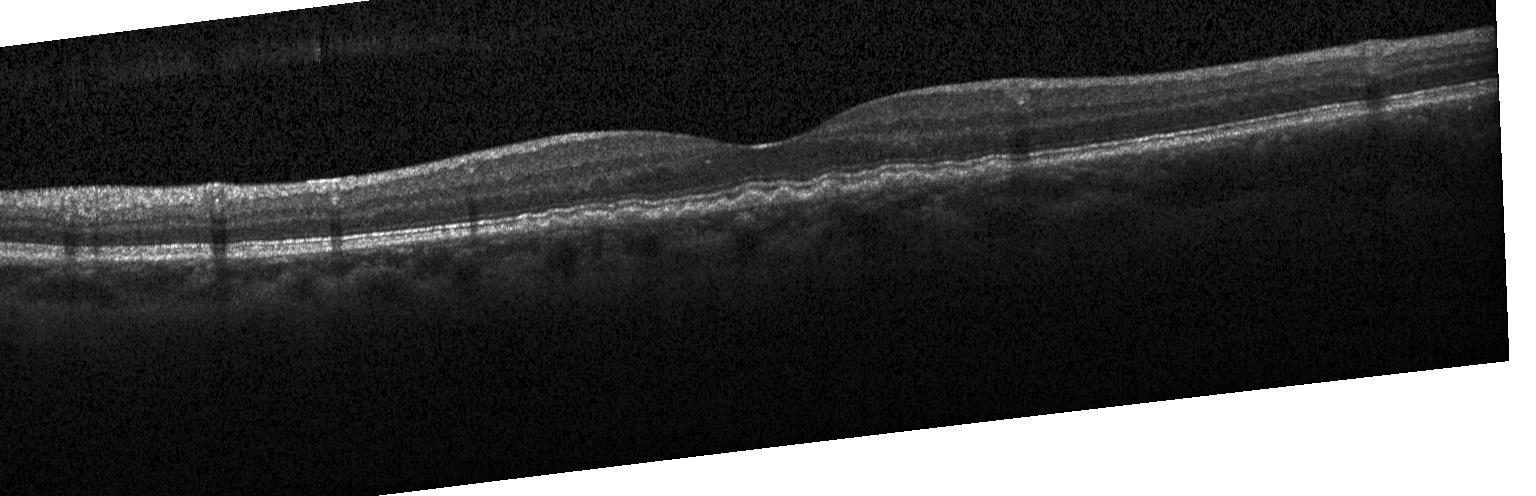
Optical coherence tomography scan.
Assessment: drusen.